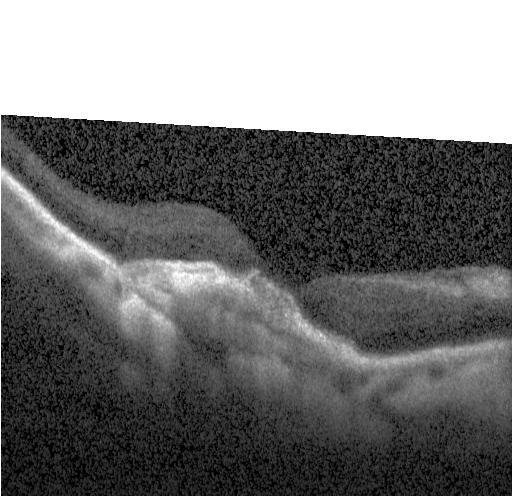 Retinal OCT B-scan — This B-scan demonstrates a choroidal neovascular membrane.